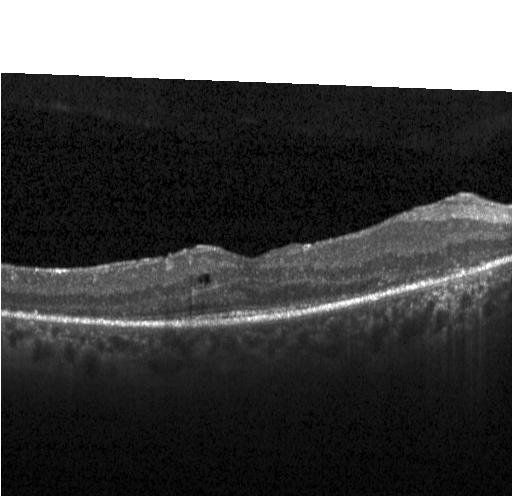
Horizontal scan through the fovea. OCT B-scan.
This B-scan demonstrates diabetic macular edema (DME).